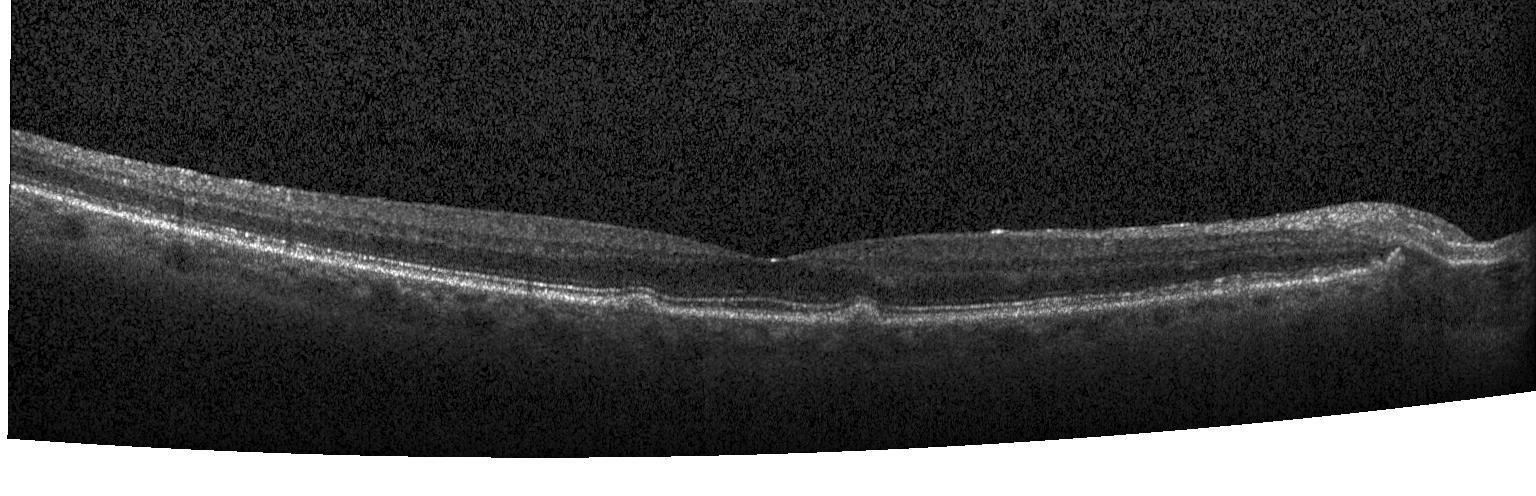 Retinal OCT cross-section; spectral-domain OCT; instrument: Heidelberg Spectralis; horizontal scan through the fovea — Multiple drusen.